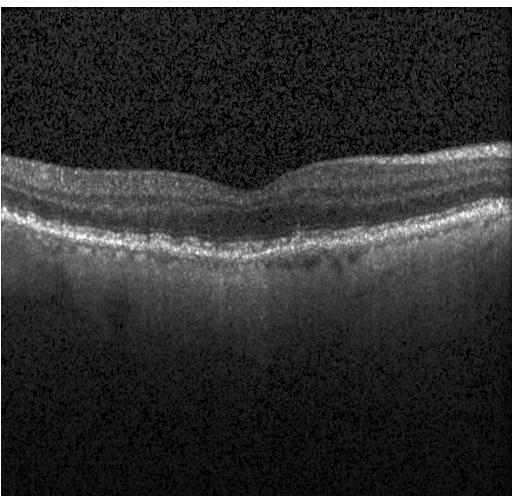

SD-OCT. Instrument: Heidelberg Spectralis. Retinal OCT B-scan. Impression: sub-RPE drusenoid deposits.